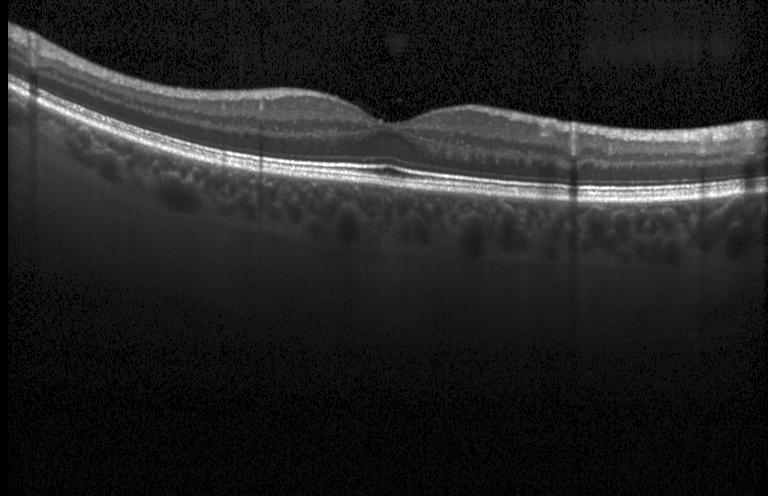
OCT B-scan. Heidelberg Spectralis. Macular OCT: no choroidal neovascularization, no diabetic macular edema, and no drusen.